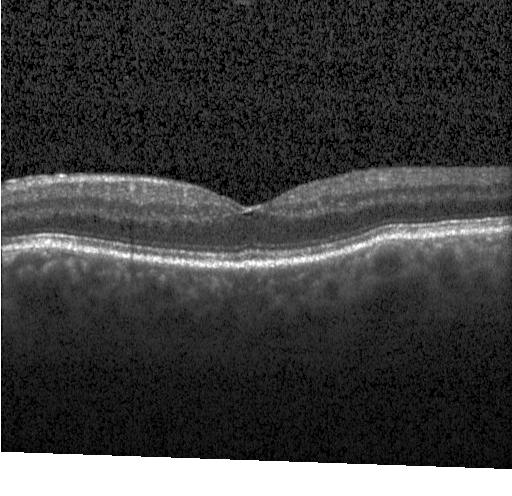
Retinal OCT cross-section
Macular OCT: no evidence of choroidal neovascularization, diabetic macular edema, or drusen.